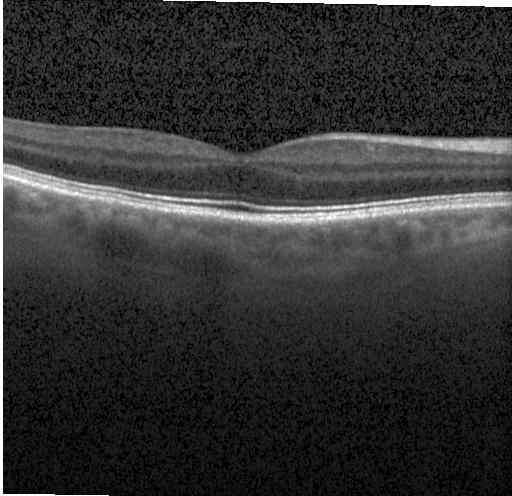
Spectral-domain OCT · retinal OCT B-scan.
Impression: no choroidal neovascularization, no diabetic macular edema, and no drusen.